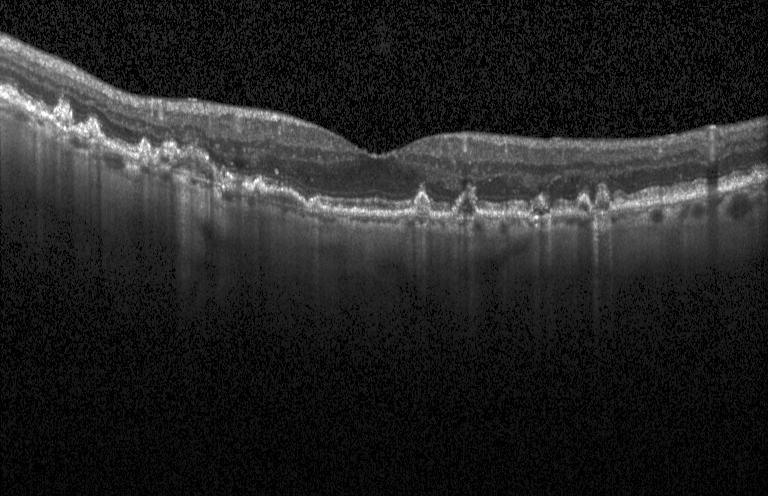

OCT B-scan — Diagnosis: a choroidal neovascular membrane.